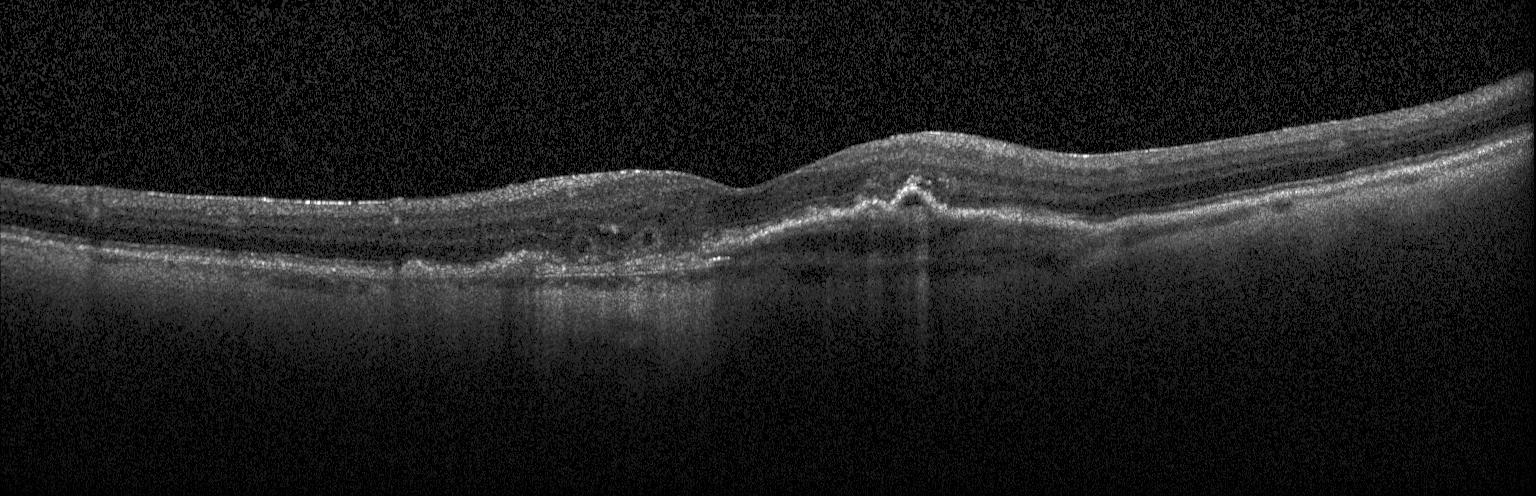 OCT line scan · Heidelberg Spectralis OCT system · spectral-domain OCT · centered on the fovea. Diagnosis: choroidal neovascularization (CNV).